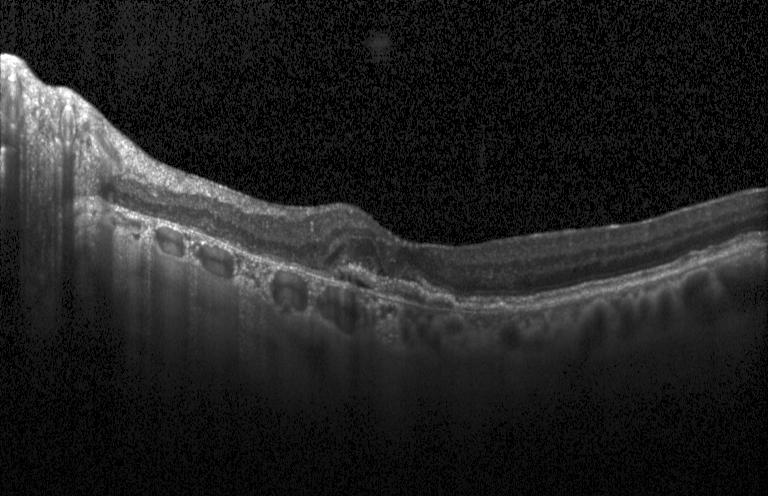

Diagnosis: a choroidal neovascular membrane.